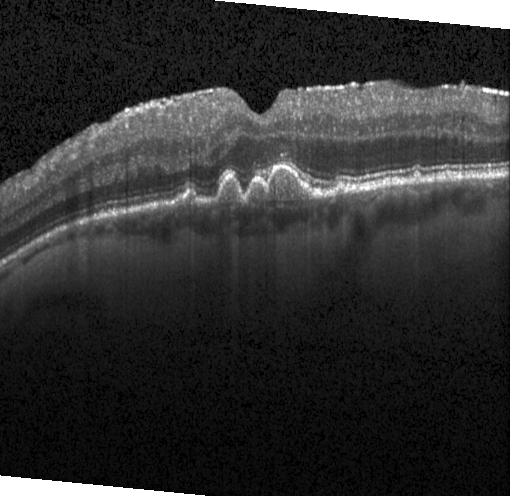 Spectral-domain OCT B-scan: sub-RPE drusenoid deposits.